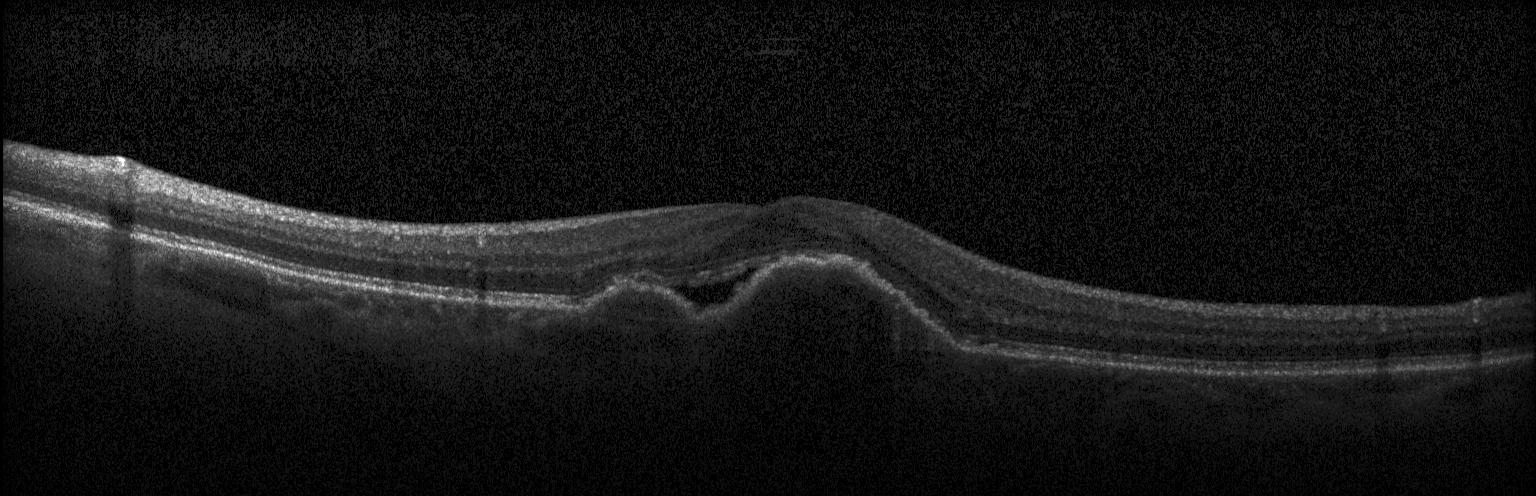 OCT line scan. Through the macula. SD-OCT. Impression: a choroidal neovascular membrane.